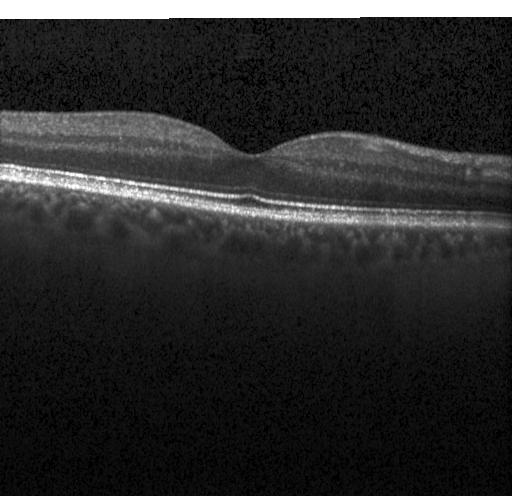 Spectral-domain OCT, retinal OCT B-scan, horizontal scan through the fovea. No evidence of CNV, DME, or drusen.